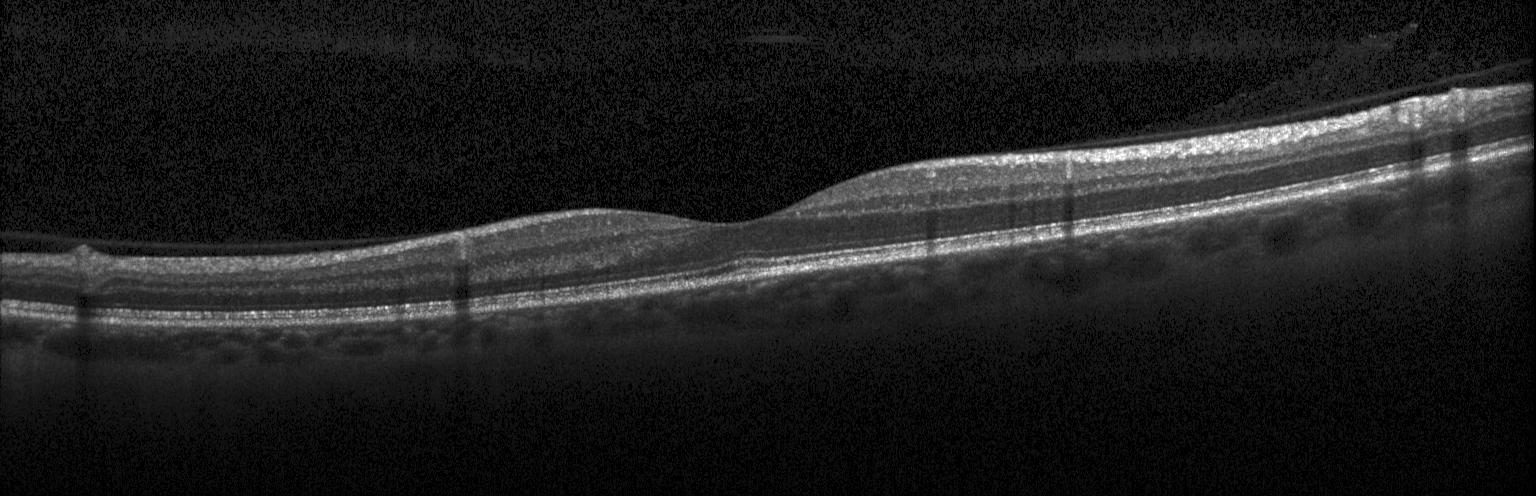
Centered on the fovea; OCT line scan
Dx: no choroidal neovascularization, diabetic macular edema, or drusen.